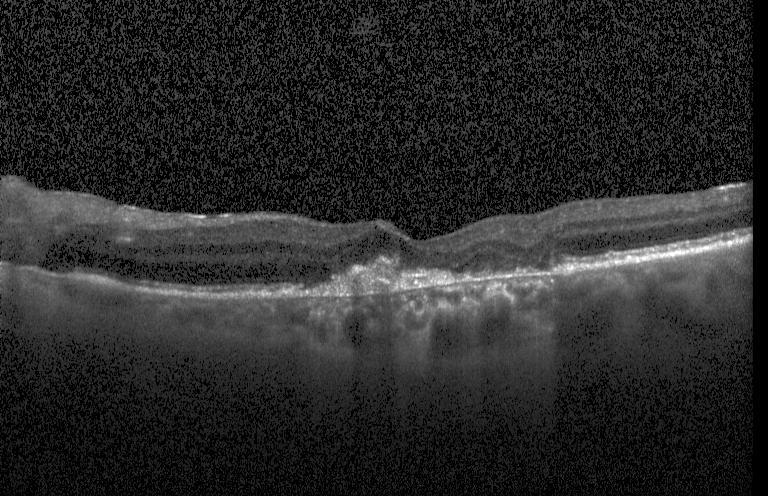
OCT B-scan; spectral-domain optical coherence tomography; fovea-centered — Finding: choroidal neovascularization.